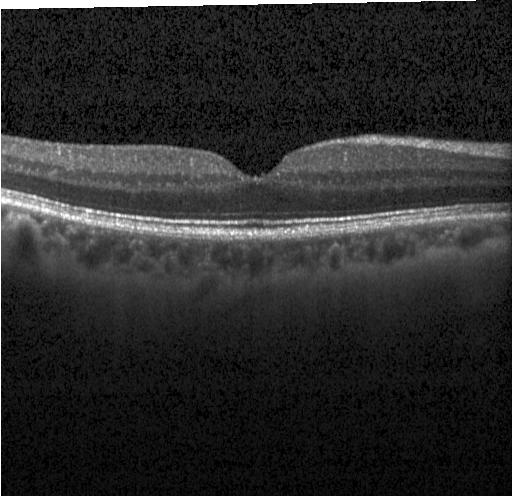 Retinal OCT cross-section. Macular OCT: no choroidal neovascularization, no diabetic macular edema, and no drusen.